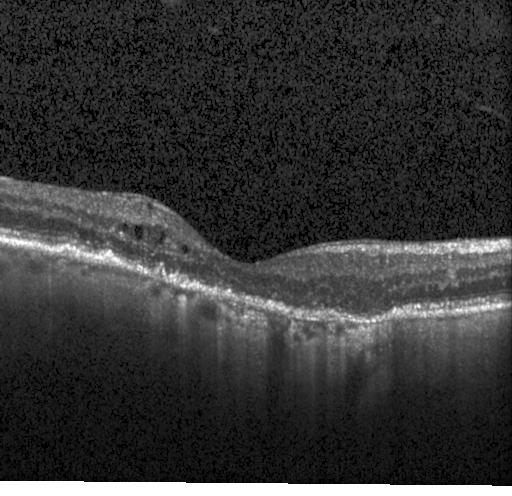 Heidelberg Spectralis OCT system · OCT line scan · fovea-centered.
This B-scan demonstrates CNV.